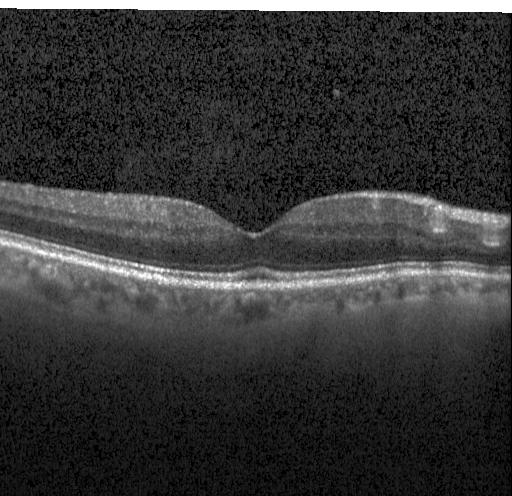
Dx: no CNV, no DME, and no drusen.